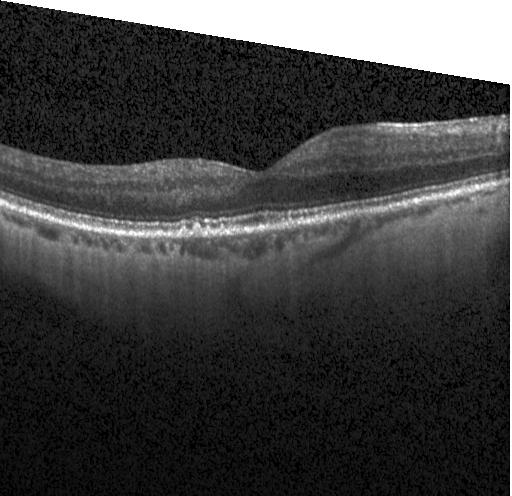

Optical coherence tomography scan. Multiple drusen.